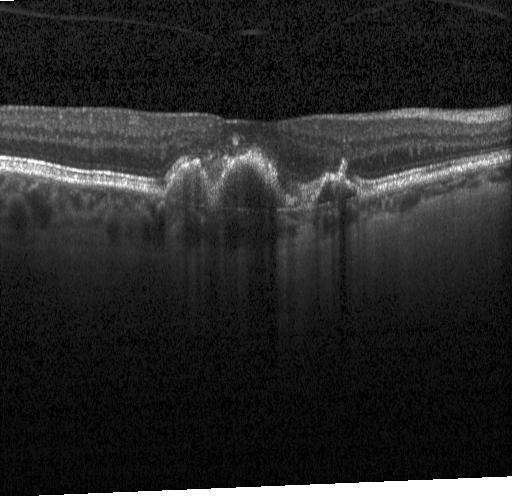

Dx: CNV.